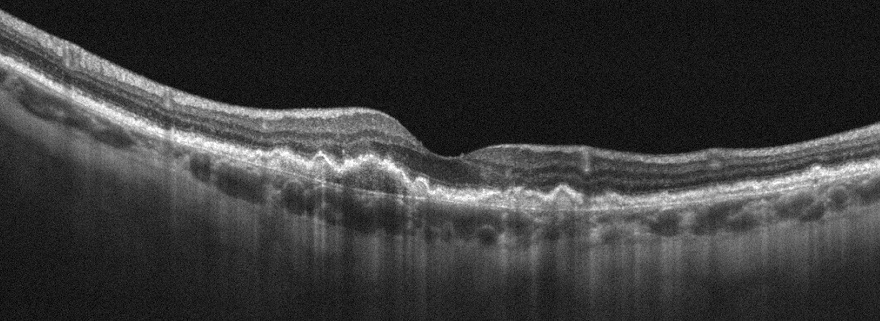

Optical coherence tomography B-scan · macular scan · instrument: Optovue Avanti RTVue XR
Assessment: AMD.